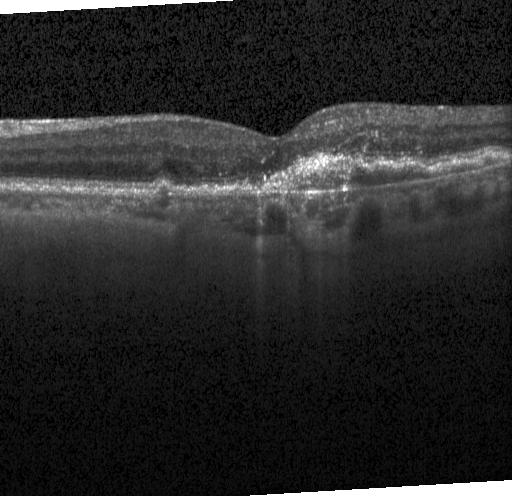

Optical coherence tomography scan, macular scan. The scan shows choroidal neovascularization (CNV).